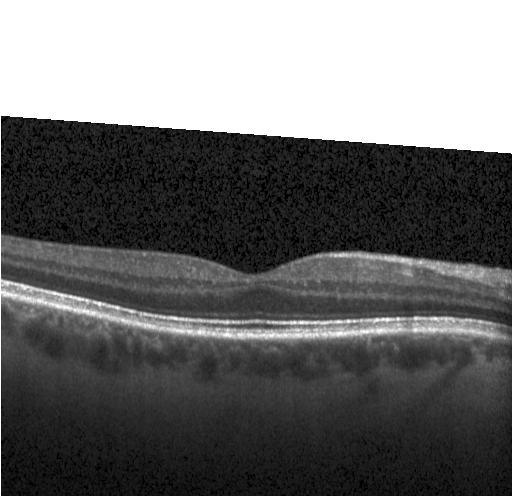 Heidelberg Spectralis · retinal OCT B-scan · SD-OCT. OCT finding: no choroidal neovascularization, no diabetic macular edema, and no drusen.